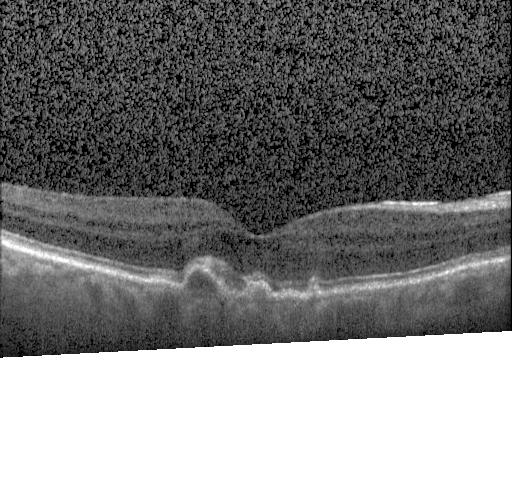
Fovea-centered; retinal OCT B-scan; spectral-domain optical coherence tomography. Impression: sub-RPE drusenoid deposits.